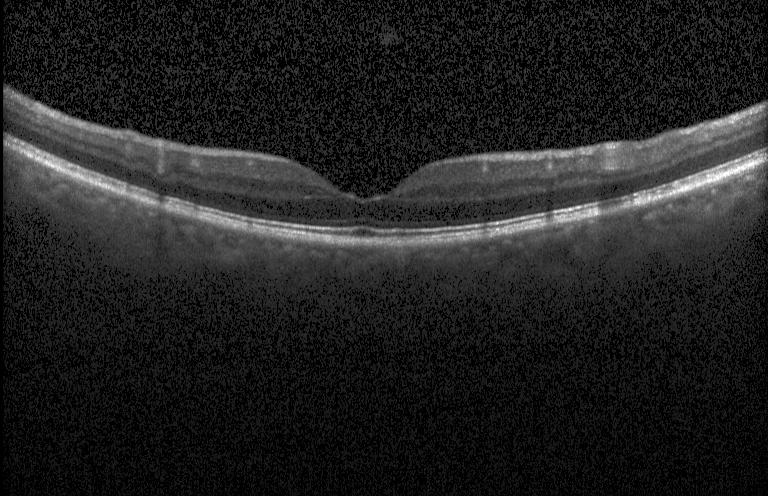

OCT B-scan, fovea-centered, instrument: Heidelberg Spectralis — Impression: no choroidal neovascularization, no diabetic macular edema, and no drusen.